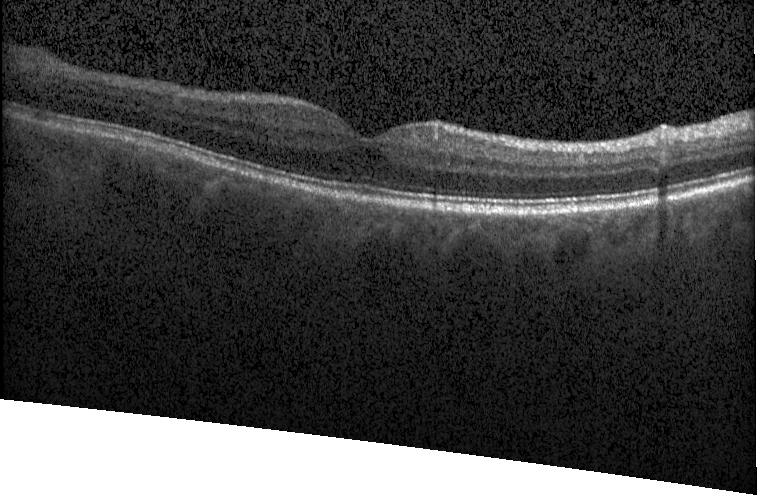

Neither CNV, DME, nor drusen.